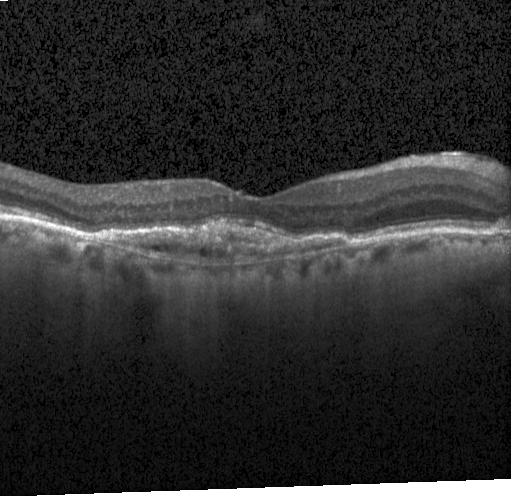
Retinal OCT cross-section showing CNV.